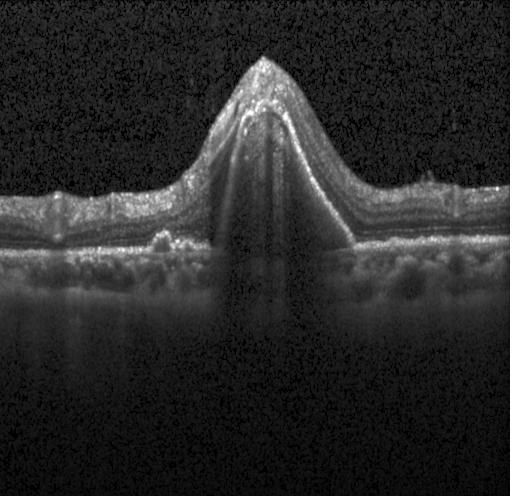
Optical coherence tomography B-scan; through the macula
Macular OCT: a choroidal neovascular membrane.